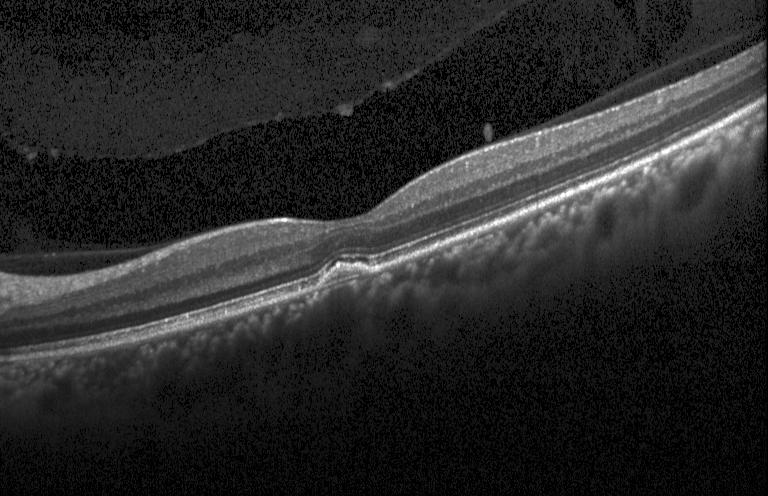 Optical coherence tomography B-scan. Acquired on a Heidelberg Spectralis. Horizontal scan through the fovea. Diagnosis: a choroidal neovascular membrane.